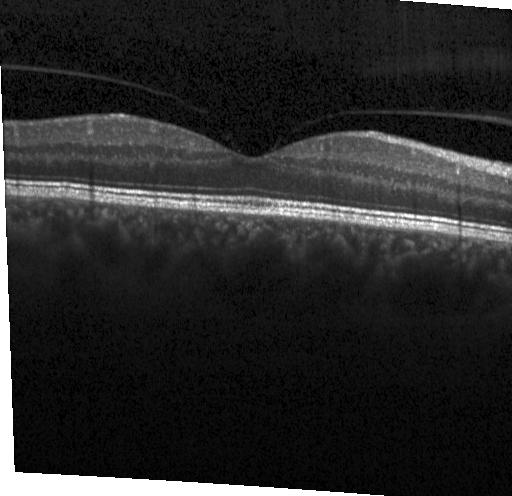

Optical coherence tomography B-scan
No CNV, no DME, and no drusen.